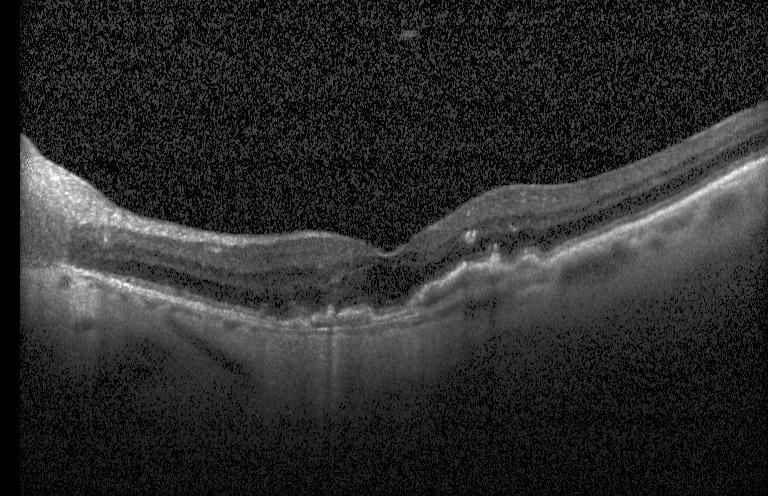
Dx: a choroidal neovascular membrane.